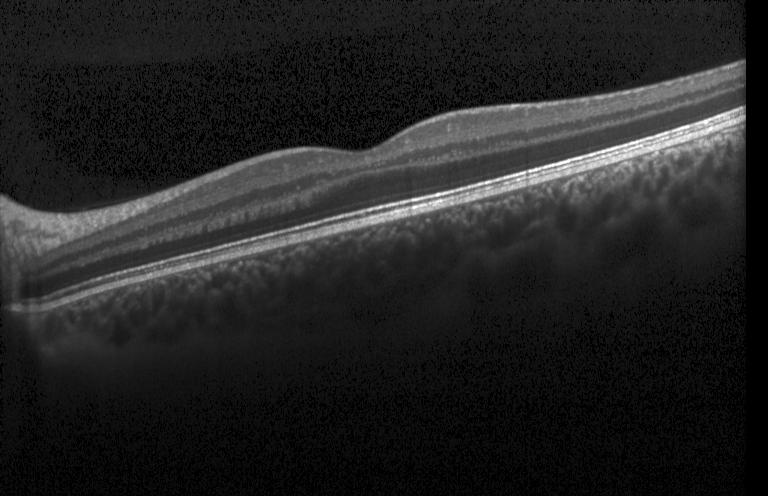 Retinal OCT cross-section; Heidelberg Spectralis; macular scan; spectral-domain optical coherence tomography.
Diagnosis: no choroidal neovascularization, no diabetic macular edema, and no drusen.